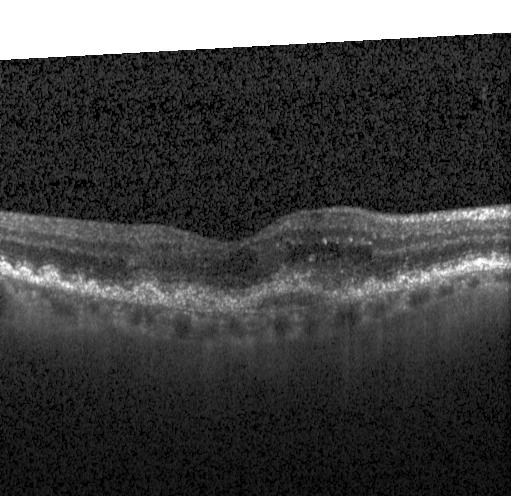
Macular OCT demonstrating a choroidal neovascular membrane.